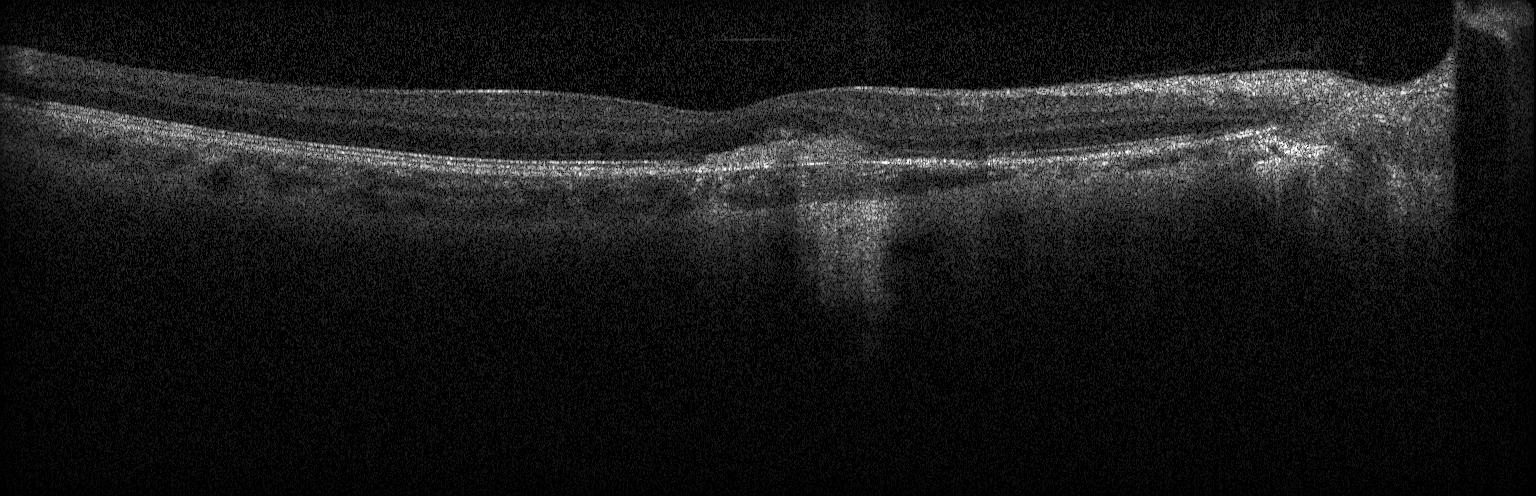 Macular OCT: choroidal neovascularization (CNV).